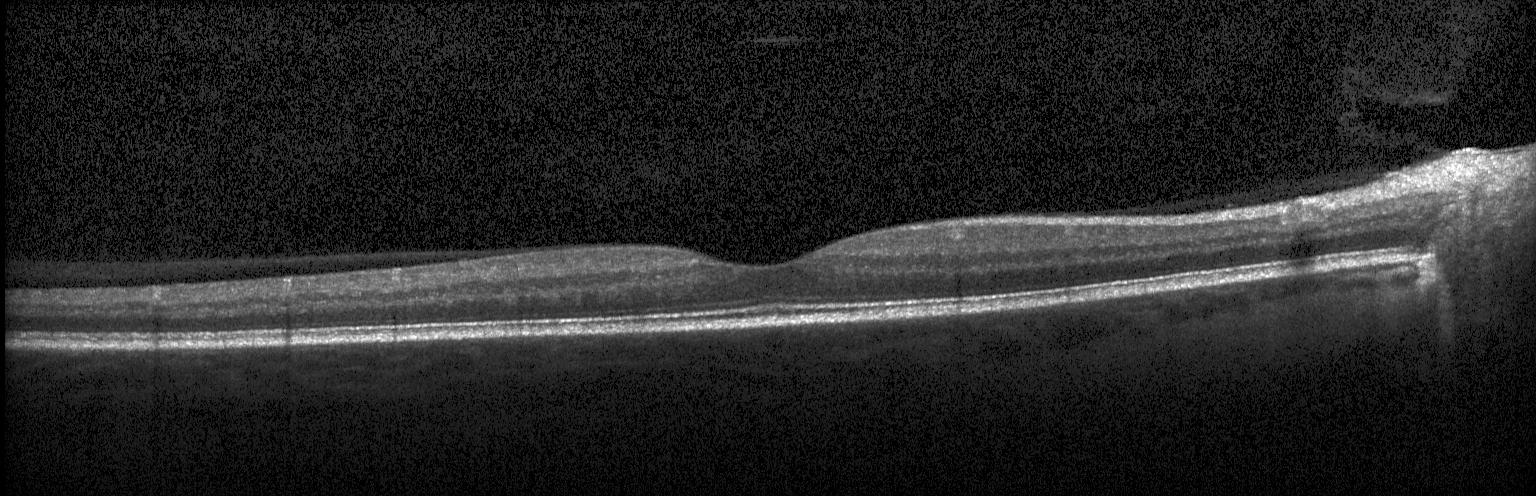 Spectral-domain OCT · horizontal scan through the fovea · retinal OCT B-scan
Impression: neither choroidal neovascularization, diabetic macular edema, nor drusen.